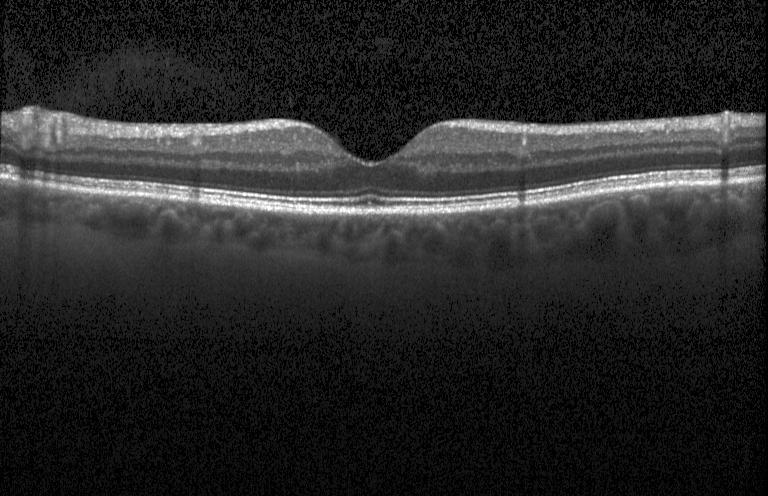 SD-OCT. Retinal OCT B-scan. Instrument: Heidelberg Spectralis.
Finding: no choroidal neovascularization, no diabetic macular edema, and no drusen.